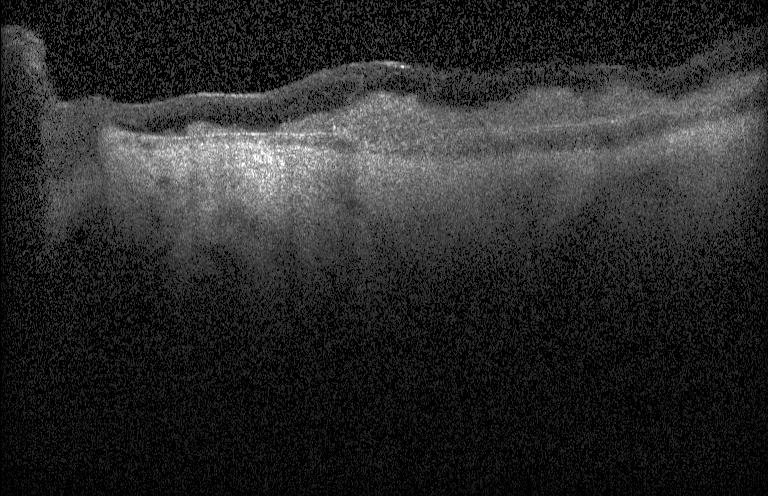
Fovea-centered. Heidelberg Spectralis. Spectral-domain optical coherence tomography. OCT B-scan — Finding: a choroidal neovascular membrane.